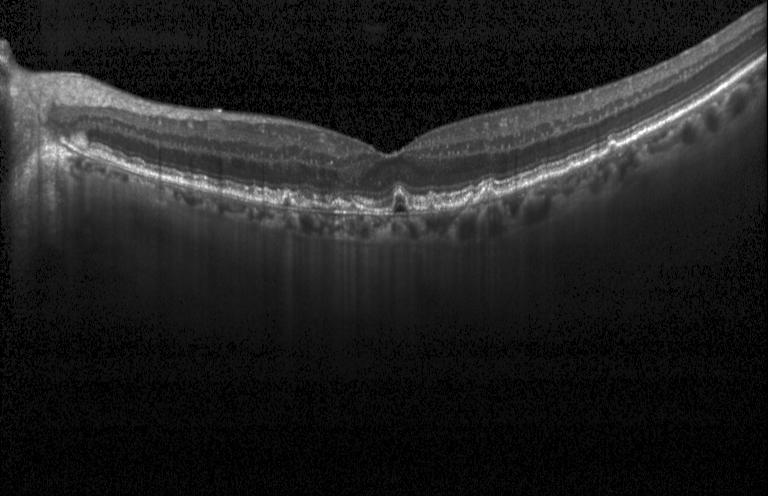 Retinal OCT cross-section showing drusen.